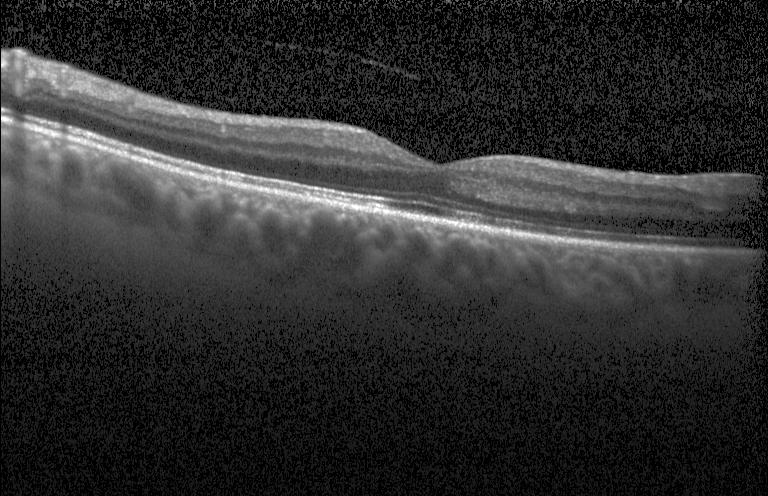 Diagnosis: neither choroidal neovascularization, diabetic macular edema, nor drusen.